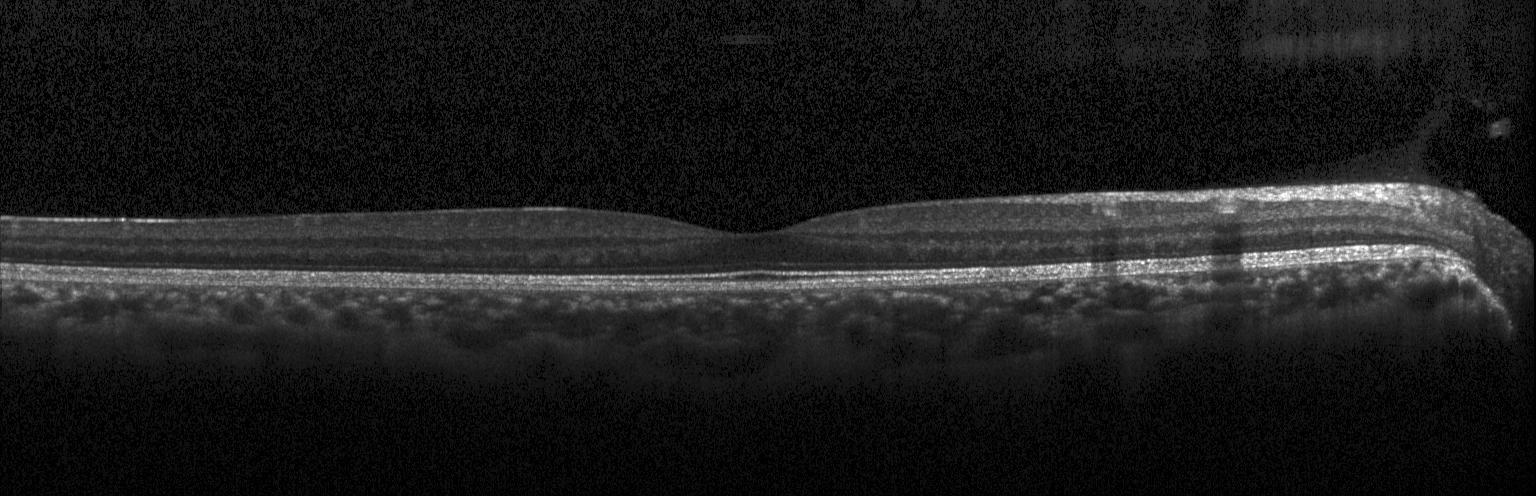

Retinal OCT B-scan, centered on the fovea.
This B-scan demonstrates no CNV, no DME, and no drusen.